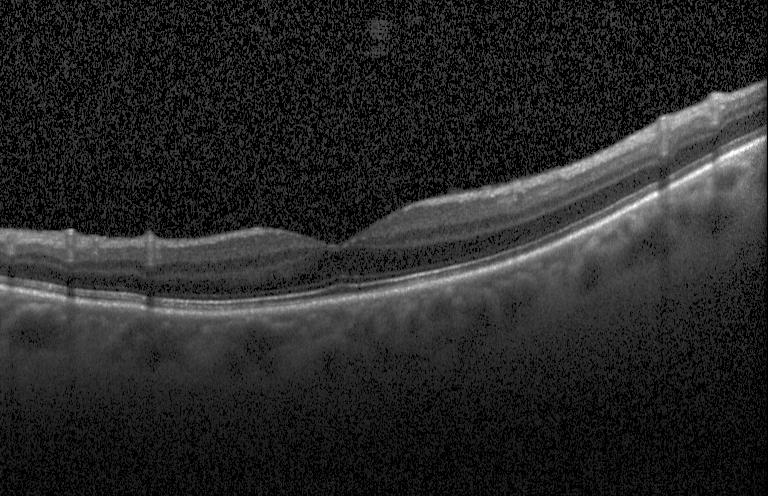 Assessment: neither CNV, DME, nor drusen.